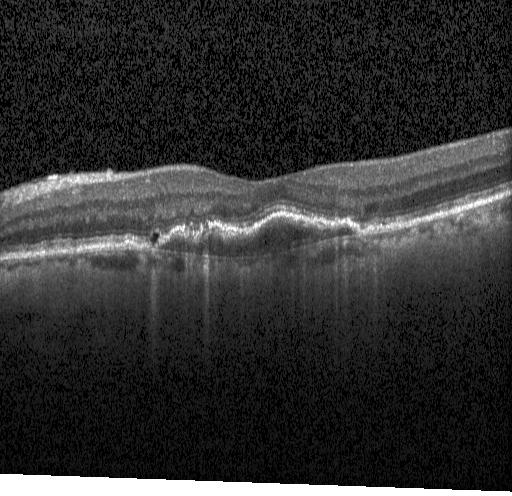 OCT line scan · through the macula.
Impression: a choroidal neovascular membrane.